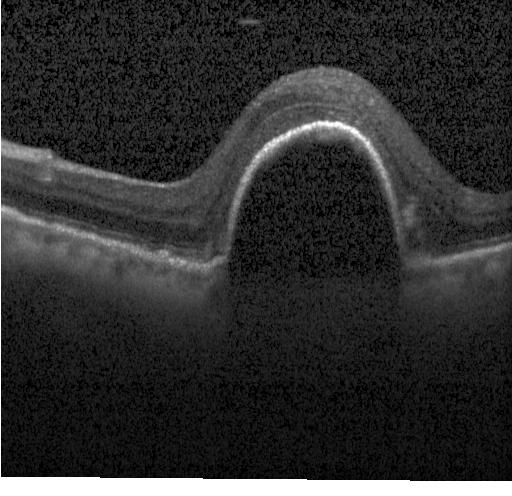
CNV.